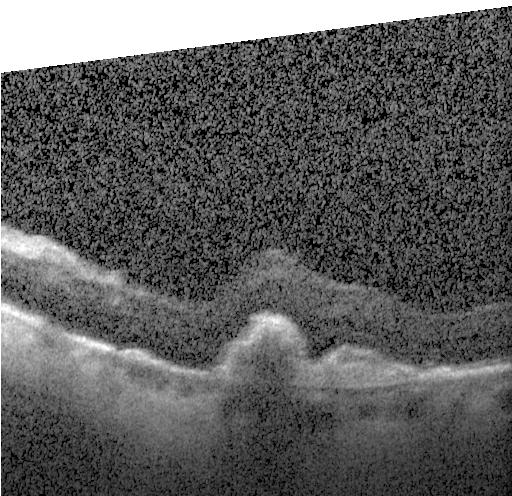

Diagnosis: a choroidal neovascular membrane.